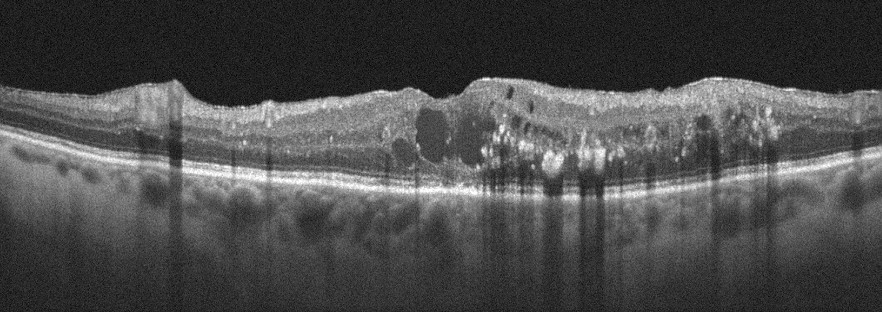
Optovue Avanti RTVue XR, optical coherence tomography B-scan, through the macula. This B-scan demonstrates diabetic macular edema (DME).